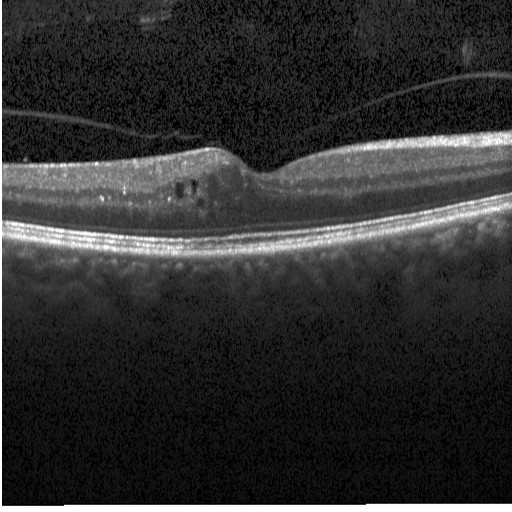

Heidelberg Spectralis OCT system, spectral-domain OCT, centered on the fovea, OCT line scan. Impression: DME.